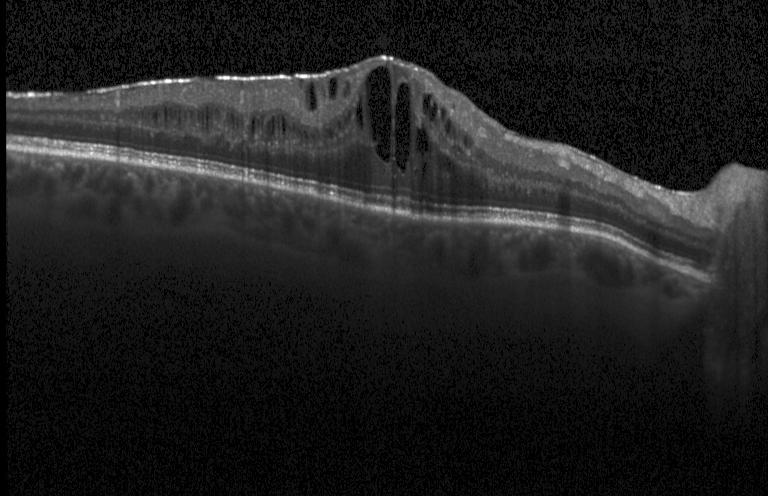 Impression: DME.